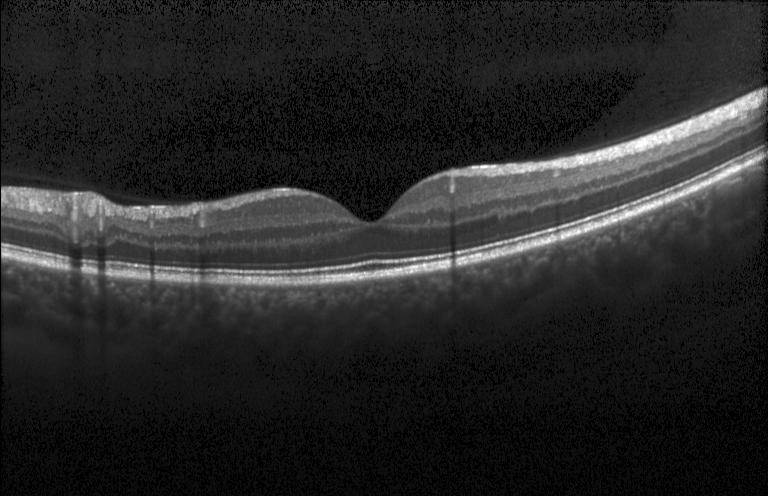

Macular OCT demonstrating no evidence of CNV, DME, or drusen.